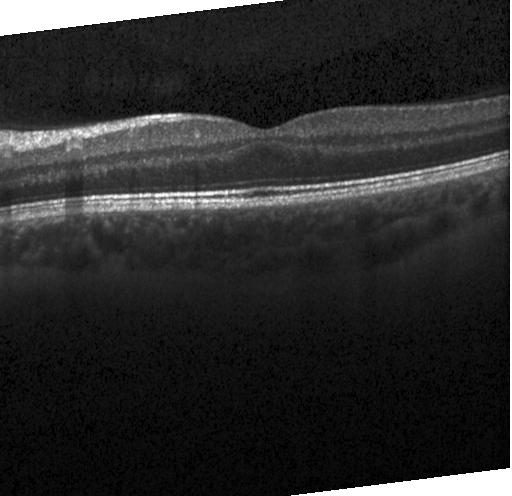

The scan shows neither choroidal neovascularization, diabetic macular edema, nor drusen.